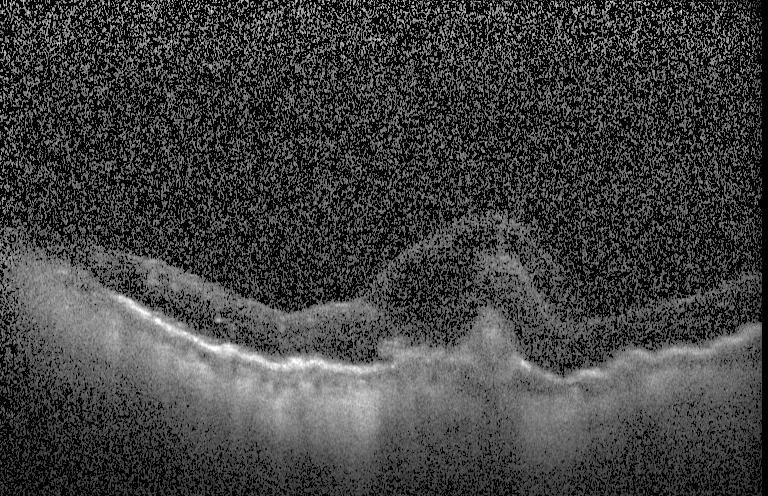
Finding: choroidal neovascularization (CNV).